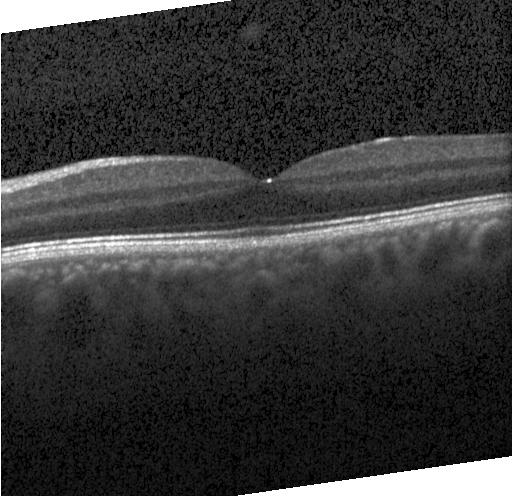
OCT B-scan; centered on the fovea.
The scan shows no CNV, DME, or drusen.